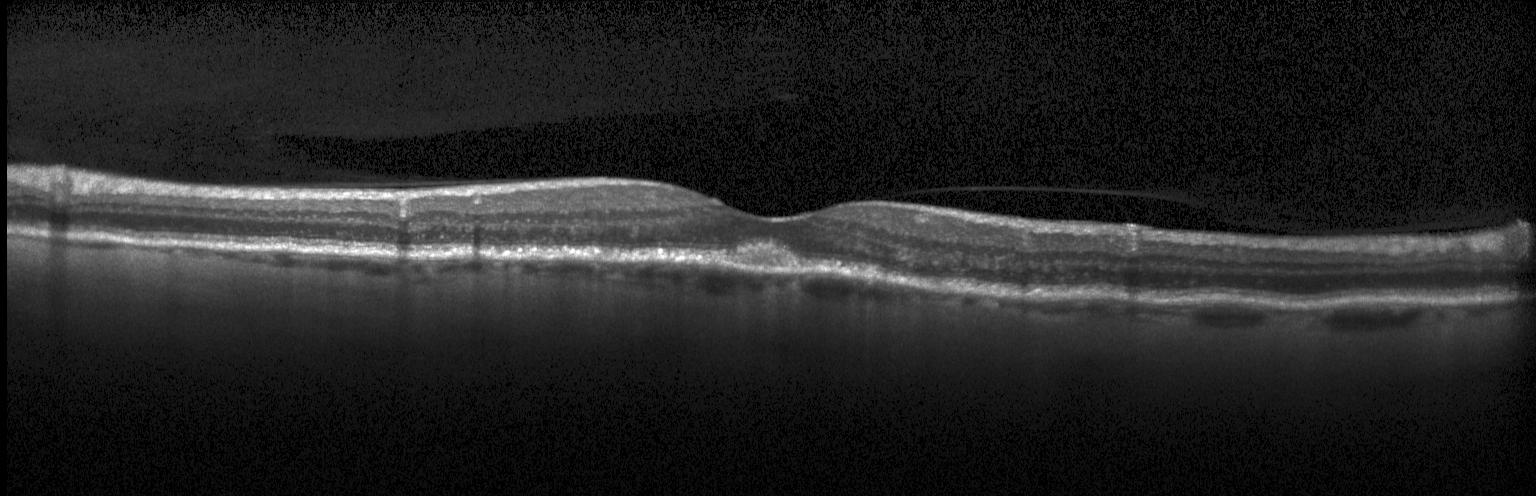

Diagnosis: multiple drusen.